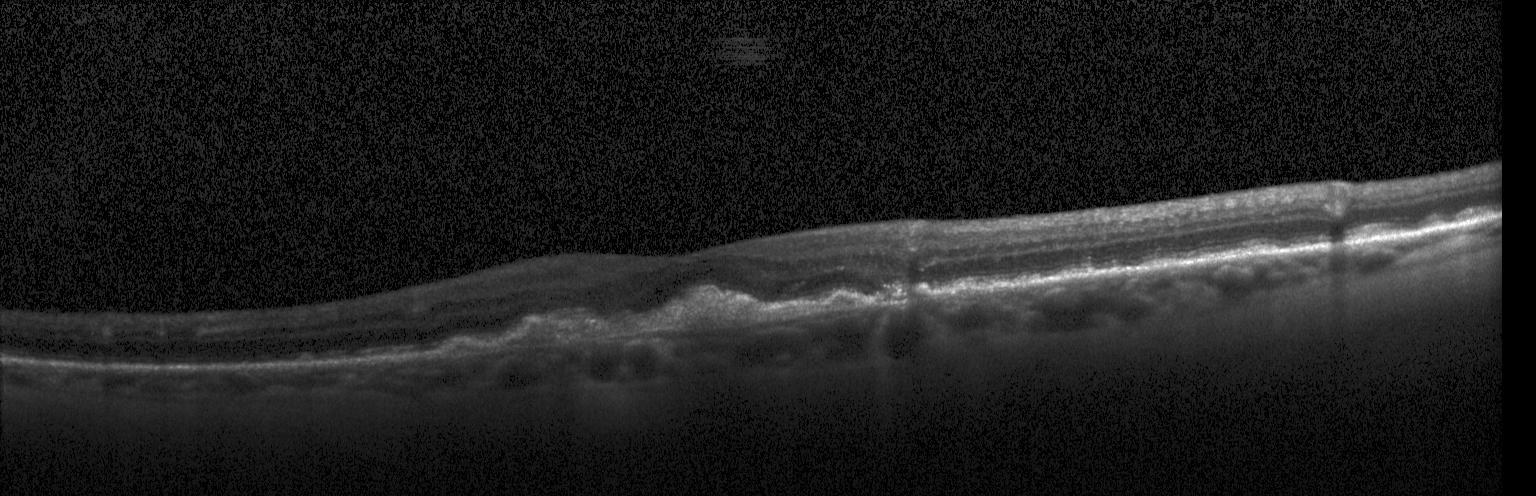
Impression: choroidal neovascularization.